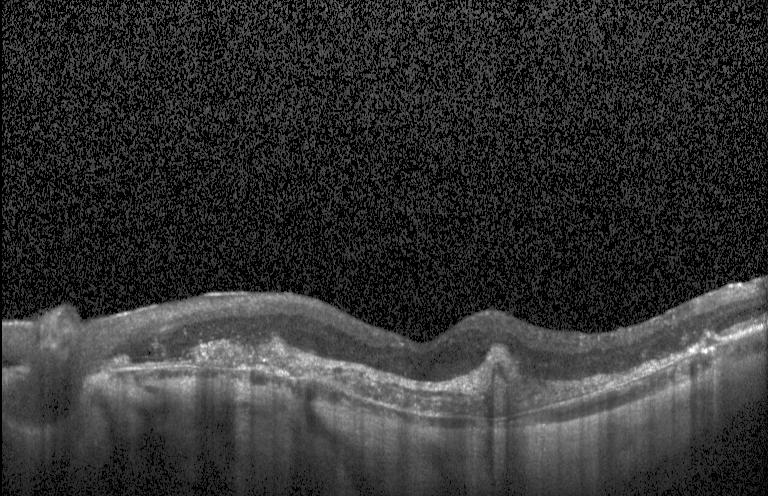
Centered on the fovea, optical coherence tomography B-scan
Dx: a choroidal neovascular membrane.